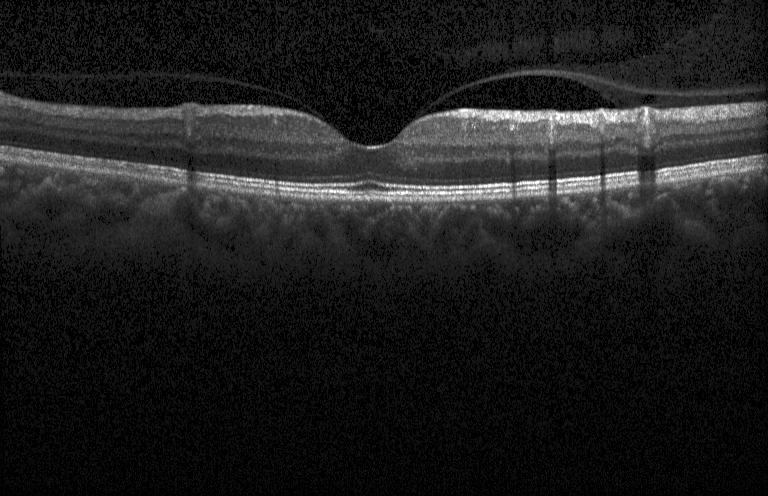 OCT B-scan · spectral-domain OCT · through the macula. Macular OCT: neither choroidal neovascularization, diabetic macular edema, nor drusen.